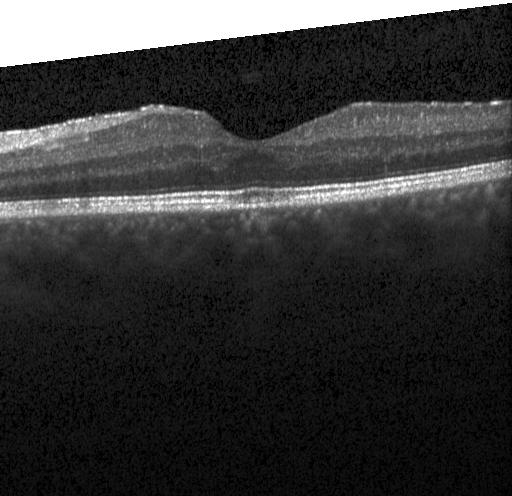
Impression: no CNV, no DME, and no drusen.